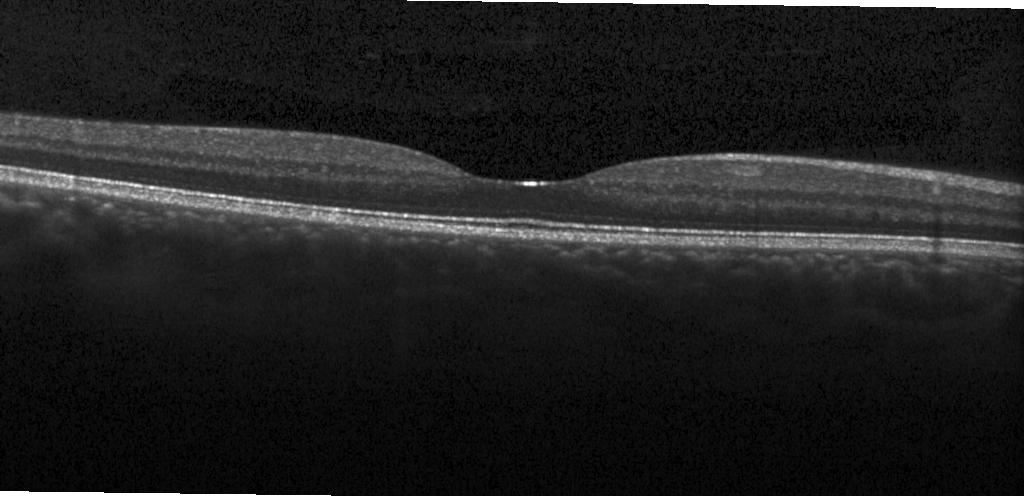

Retinal OCT cross-section
Assessment: no CNV, no DME, and no drusen.